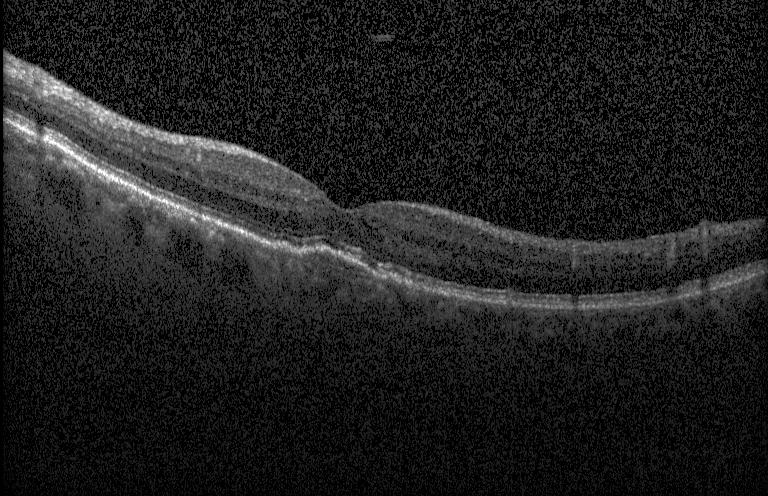
OCT line scan. This B-scan demonstrates choroidal neovascularization (CNV).